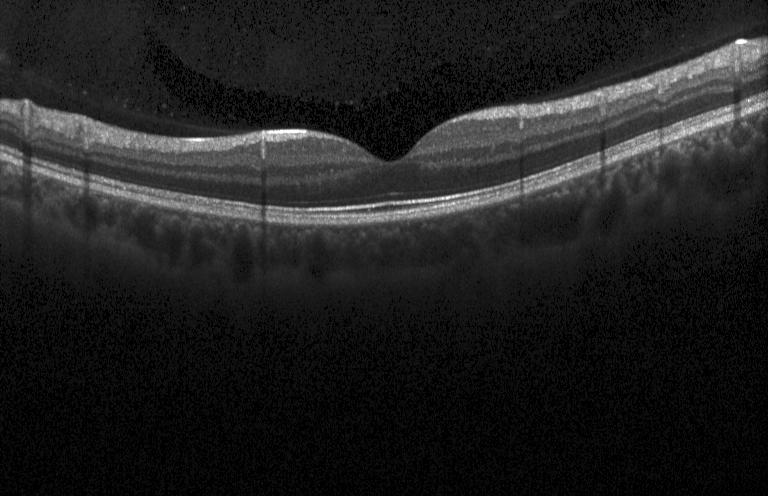

Acquired on a Heidelberg Spectralis. Optical coherence tomography B-scan — Impression: no evidence of choroidal neovascularization, diabetic macular edema, or drusen.